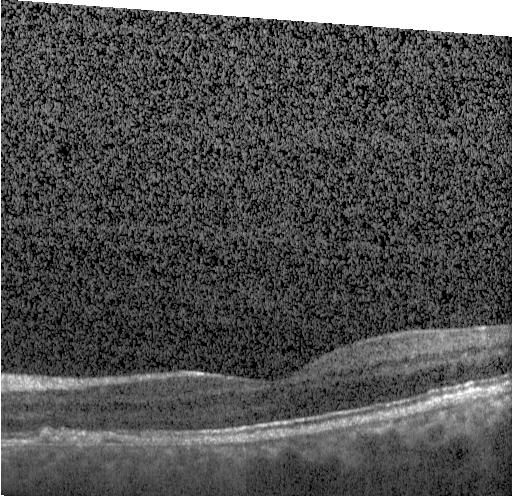
Acquired on a Heidelberg Spectralis; through the macula; spectral-domain OCT; optical coherence tomography scan — Impression: choroidal neovascularization (CNV).